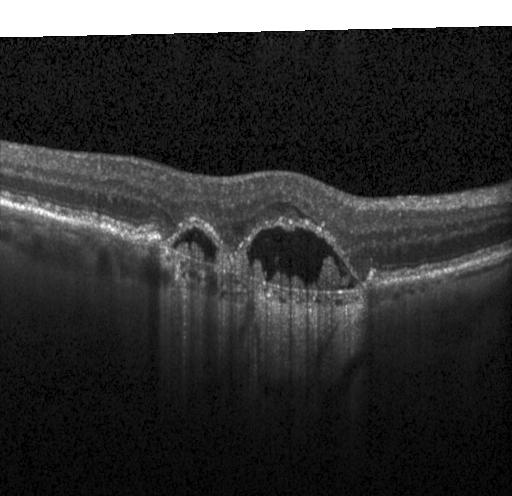

Through the macula; instrument: Heidelberg Spectralis; optical coherence tomography B-scan; spectral-domain optical coherence tomography. Impression: choroidal neovascularization (CNV).